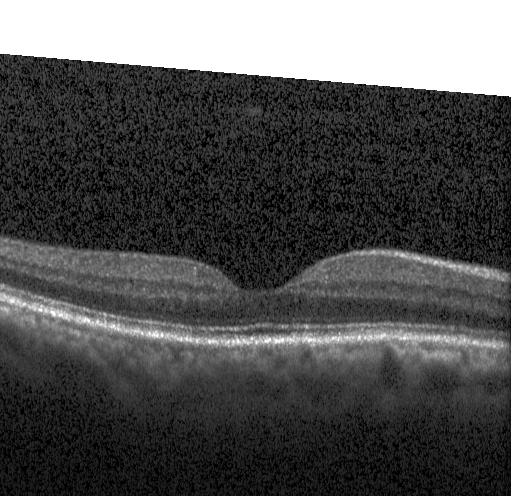 OCT line scan. This B-scan demonstrates neither choroidal neovascularization, diabetic macular edema, nor drusen.